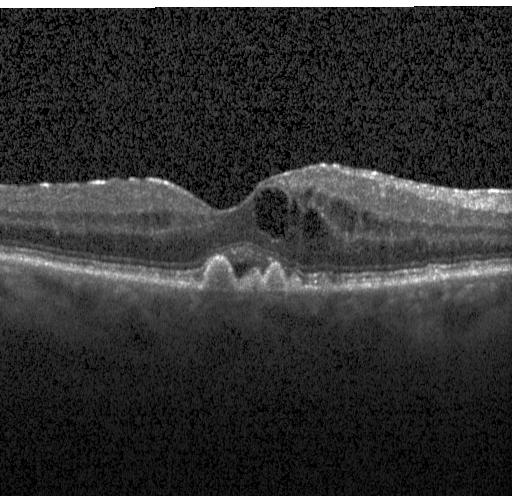 Spectral-domain optical coherence tomography; acquired on a Heidelberg Spectralis; macular scan; OCT B-scan. Finding: CNV.